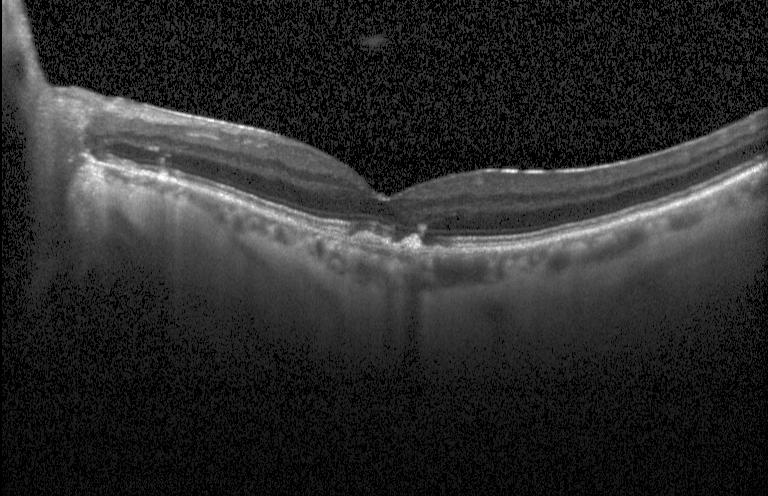
Through the macula. Retinal OCT B-scan. Instrument: Heidelberg Spectralis
Diagnosis: choroidal neovascularization.